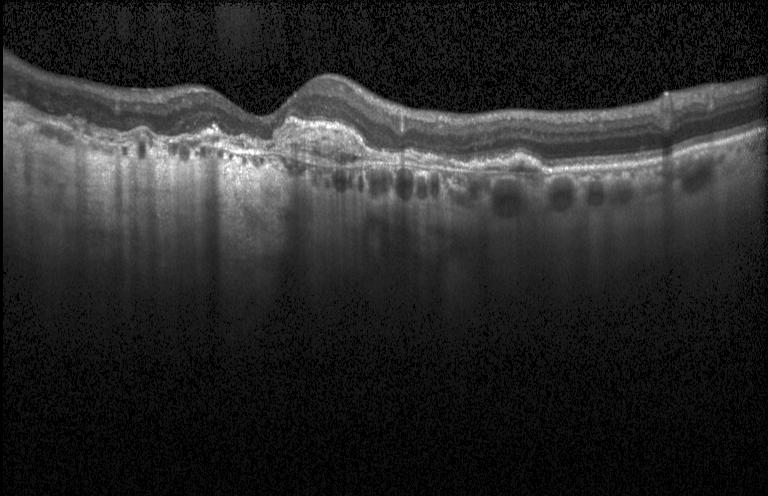 Dx: a choroidal neovascular membrane.